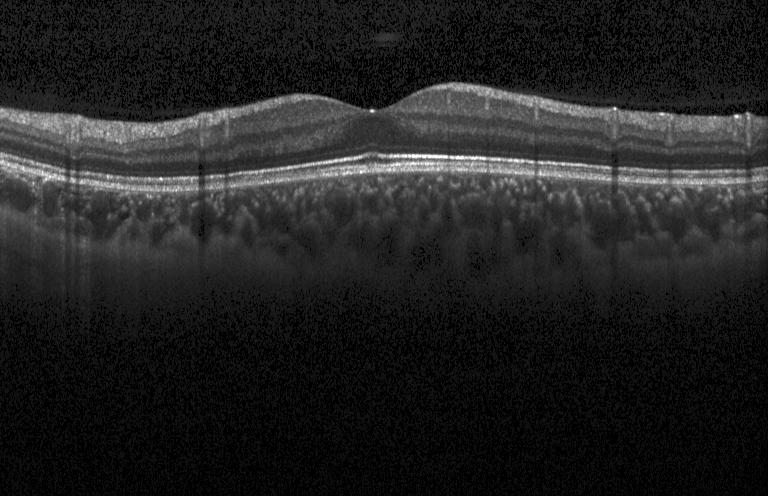
Diagnosis: no evidence of choroidal neovascularization, diabetic macular edema, or drusen.